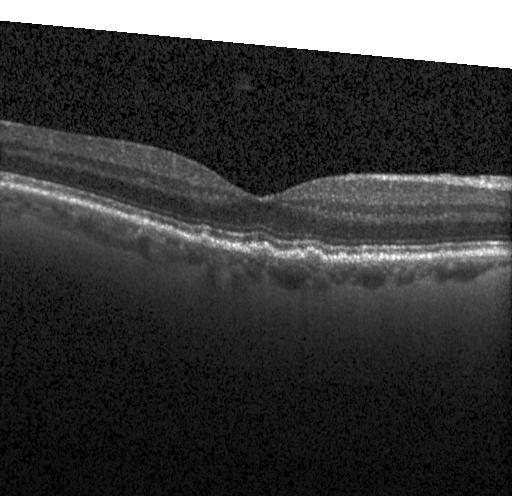 Retinal OCT cross-section. Fovea-centered. Dx: multiple drusen.